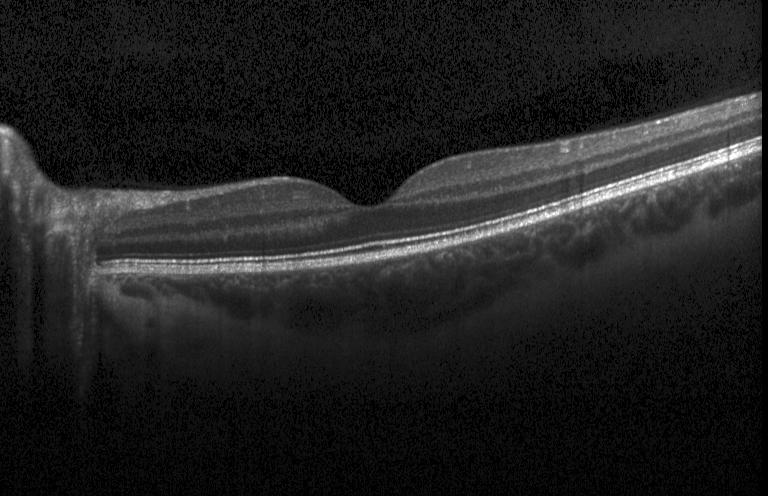

Macular OCT: no choroidal neovascularization, diabetic macular edema, or drusen.